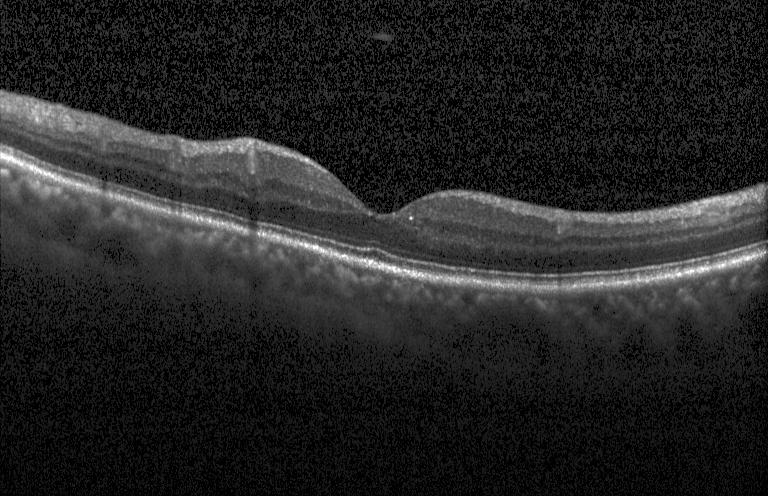 Optical coherence tomography scan. SD-OCT — Finding: no choroidal neovascularization, diabetic macular edema, or drusen.